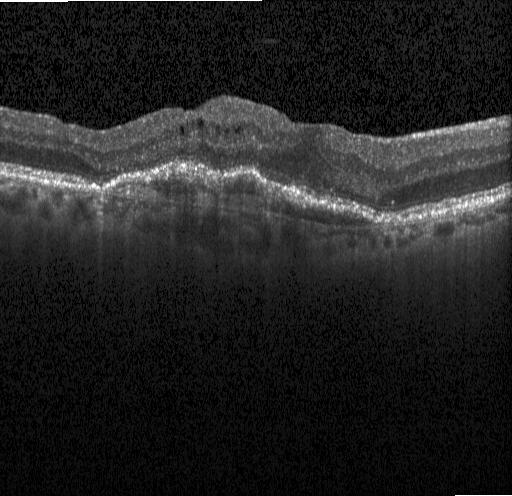
Retinal OCT B-scan; spectral-domain optical coherence tomography; Heidelberg Spectralis OCT system; centered on the fovea.
Finding: a choroidal neovascular membrane.